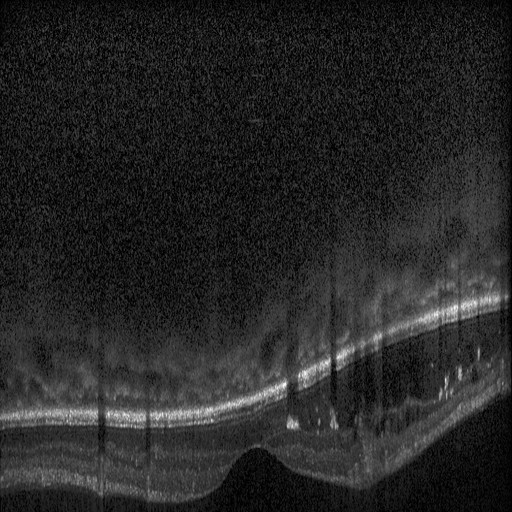
Retinal OCT cross-section showing DME.